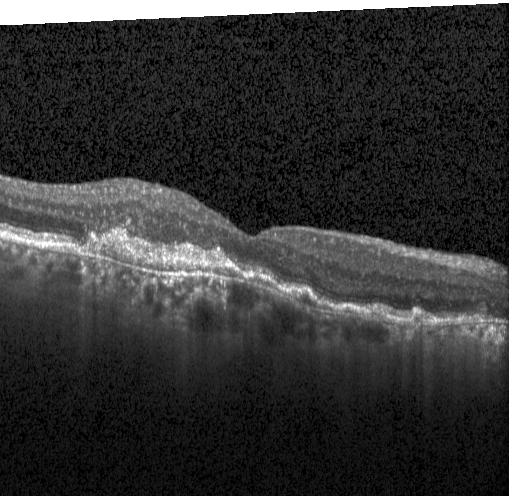
Retinal OCT B-scan. Diagnosis: a choroidal neovascular membrane.